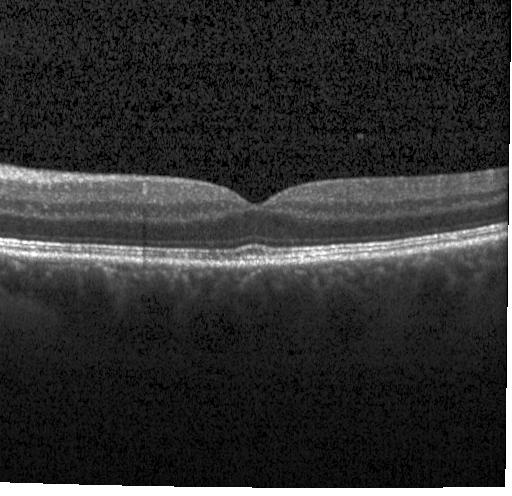 Optical coherence tomography scan, fovea-centered, spectral-domain OCT, instrument: Heidelberg Spectralis
Diagnosis: no evidence of choroidal neovascularization, diabetic macular edema, or drusen.